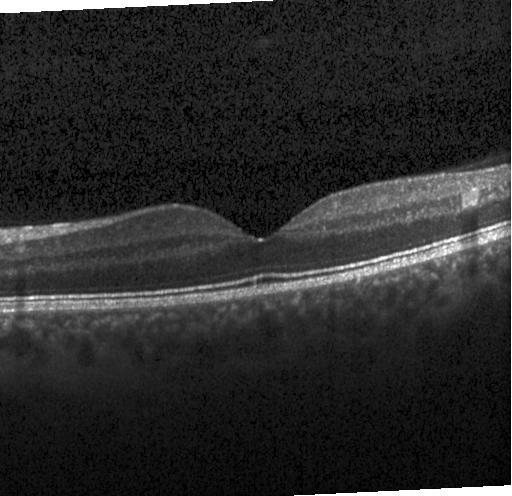 Retinal OCT cross-section, Heidelberg Spectralis OCT system — Impression: no CNV, DME, or drusen.